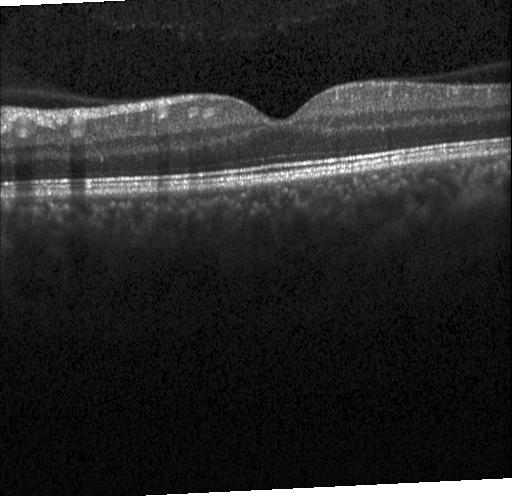
Optical coherence tomography scan, SD-OCT — Assessment: neither choroidal neovascularization, diabetic macular edema, nor drusen.